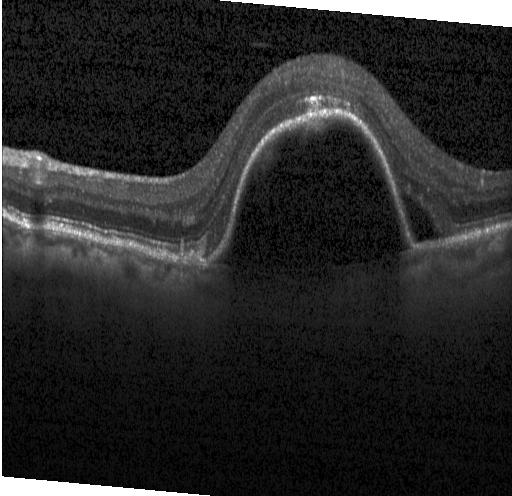
Assessment: a choroidal neovascular membrane.